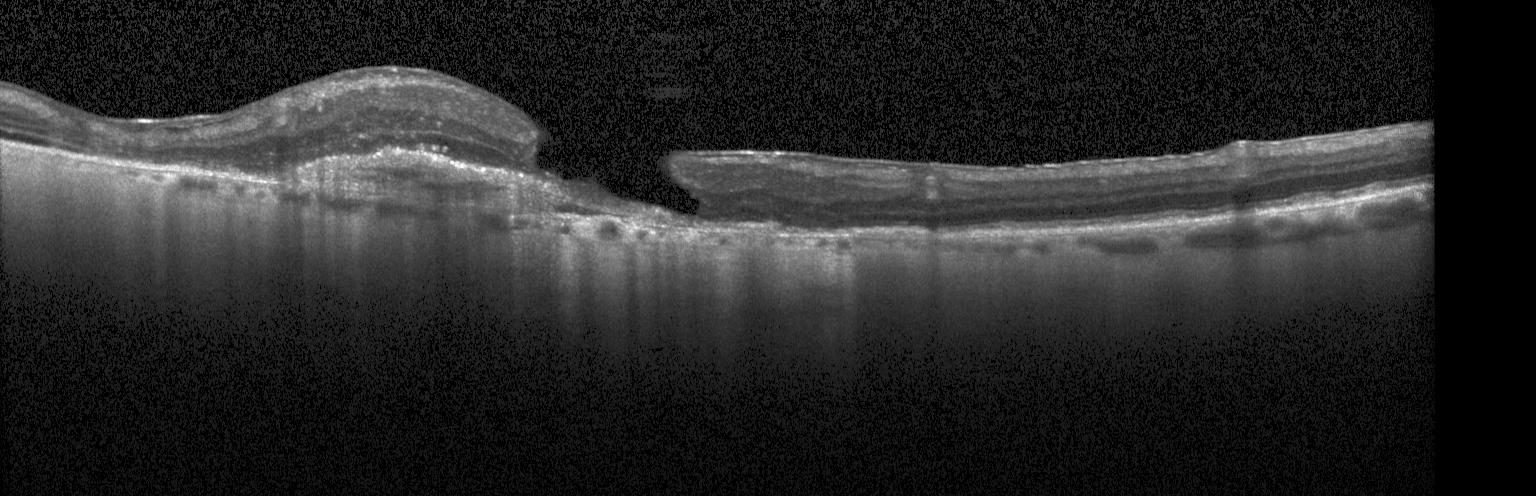 Optical coherence tomography B-scan. Acquired on a Heidelberg Spectralis
Diagnosis: CNV.